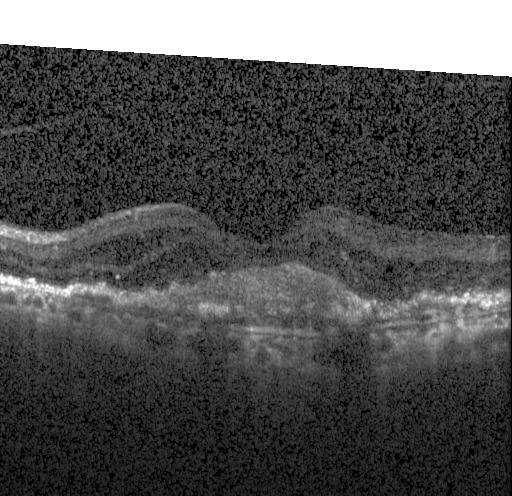 The scan shows CNV.